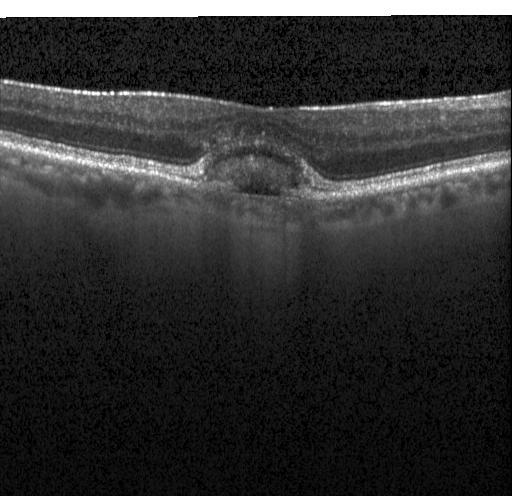

Finding: choroidal neovascularization (CNV).